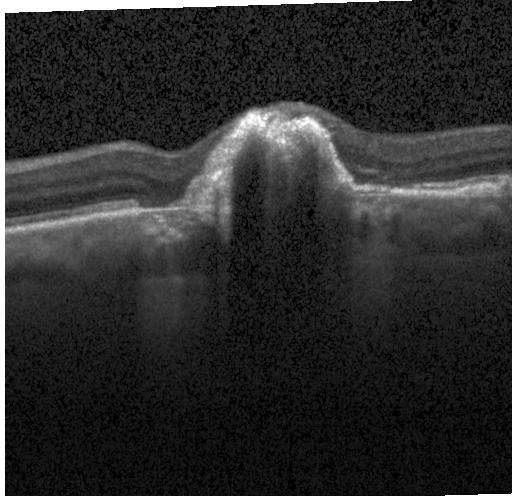

Fovea-centered · retinal OCT cross-section
Diagnosis: a choroidal neovascular membrane.